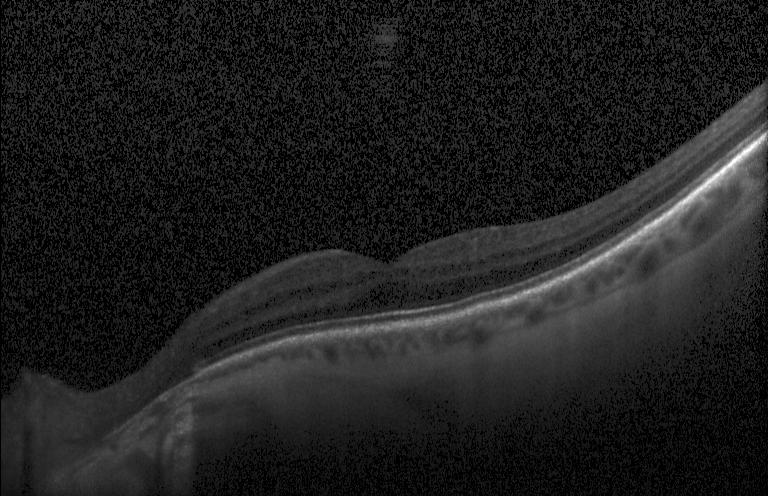

Retinal OCT cross-section showing no CNV, no DME, and no drusen.